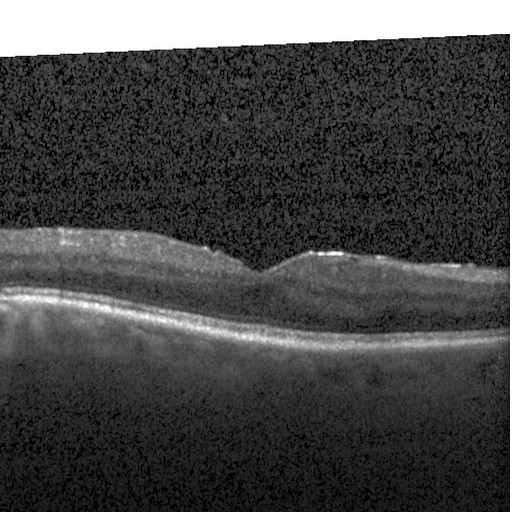 Diagnosis: diabetic macular edema.